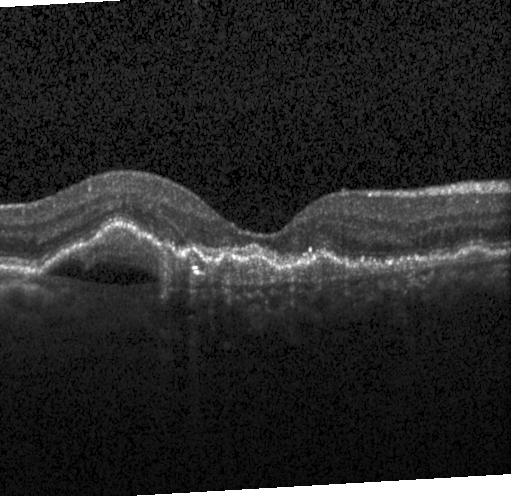

Spectral-domain OCT B-scan: a choroidal neovascular membrane.